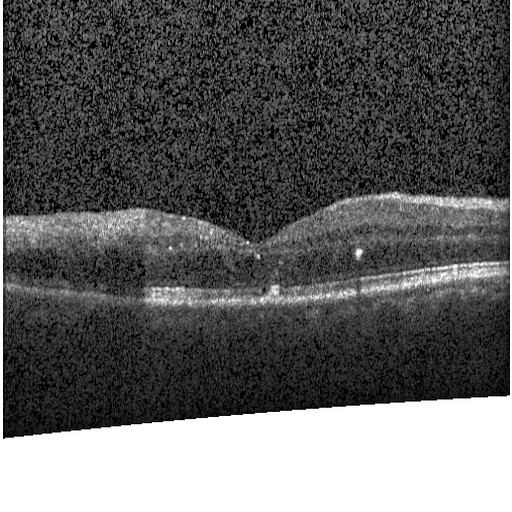
Retinal OCT cross-section; instrument: Heidelberg Spectralis — Assessment: diabetic macular edema.